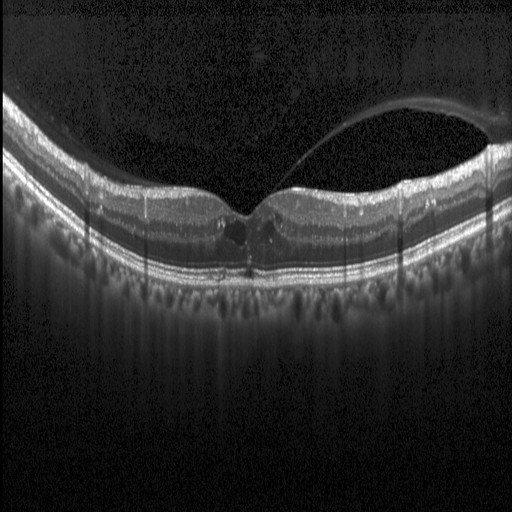 Optical coherence tomography B-scan, instrument: Heidelberg Spectralis — The scan shows DME.